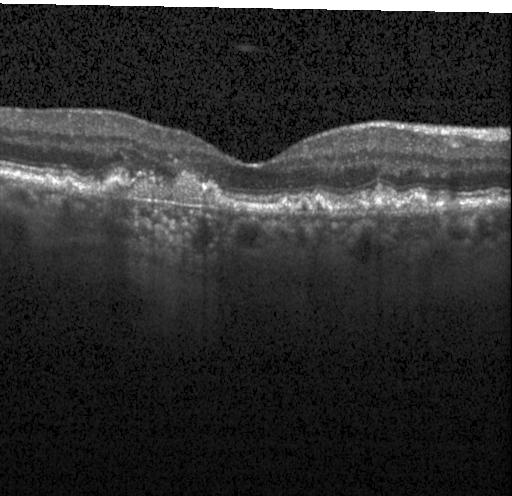
Instrument: Heidelberg Spectralis. Optical coherence tomography scan. Macular scan
Dx: a choroidal neovascular membrane.